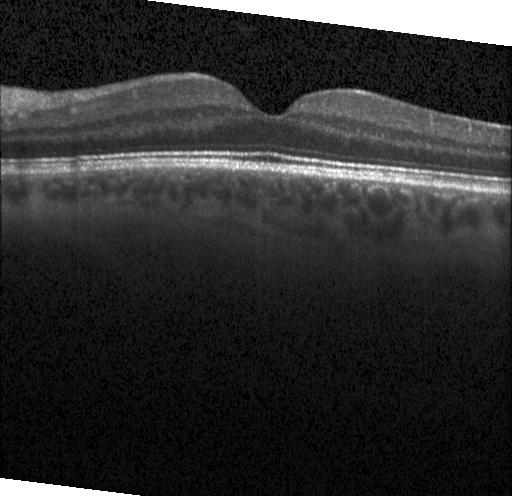

OCT scan showing no choroidal neovascularization, diabetic macular edema, or drusen.